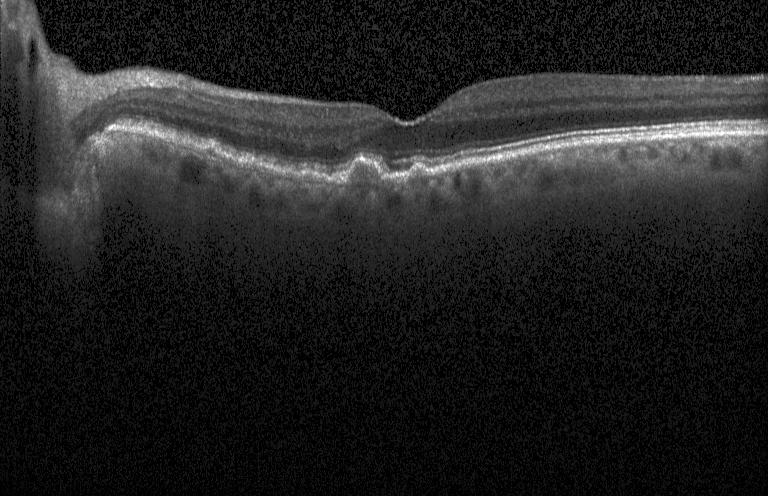
Optical coherence tomography B-scan · Heidelberg Spectralis · through the macula · SD-OCT
OCT finding: sub-RPE drusenoid deposits.